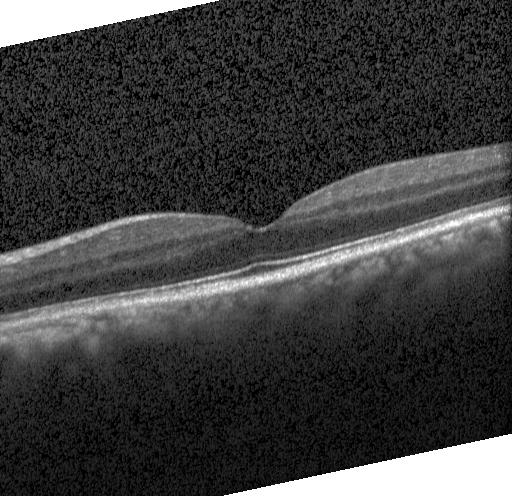
OCT line scan. The scan shows no evidence of choroidal neovascularization, diabetic macular edema, or drusen.